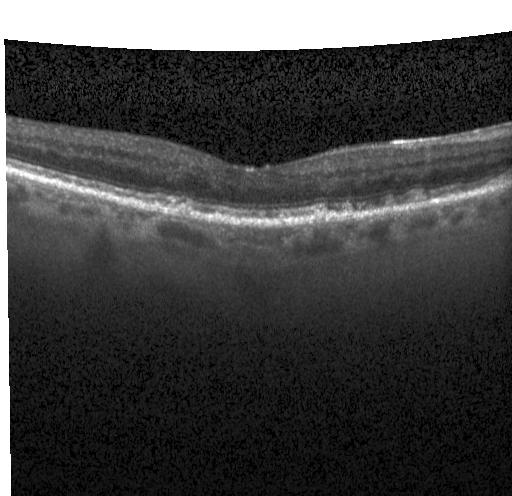 This B-scan demonstrates drusen.